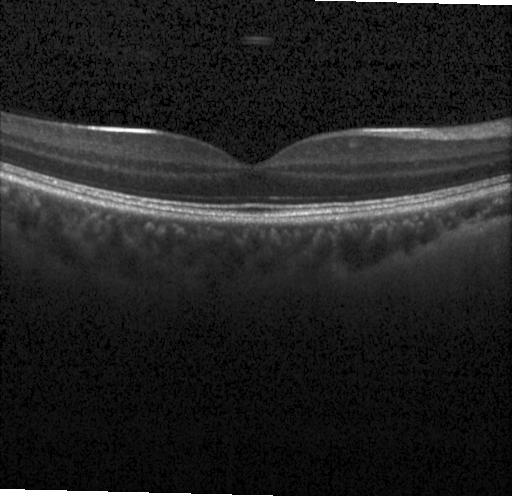

Heidelberg Spectralis OCT system · through the macula · OCT B-scan — This B-scan demonstrates no evidence of CNV, DME, or drusen.